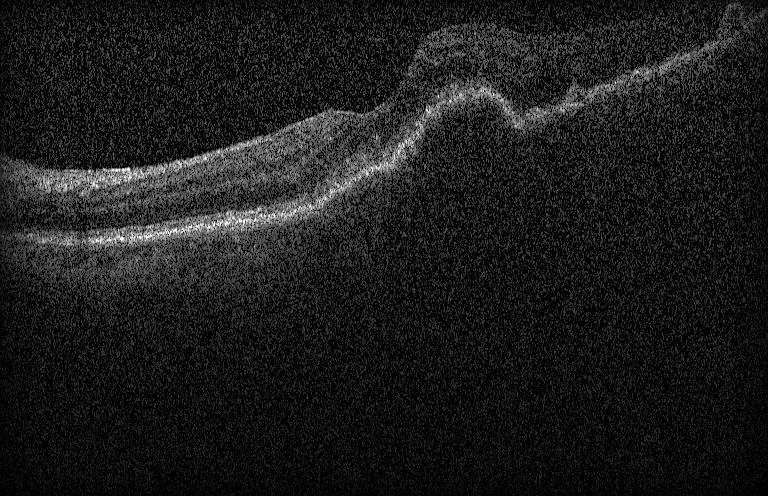
Through the macula, retinal OCT B-scan, spectral-domain OCT, acquired on a Heidelberg Spectralis. CNV.